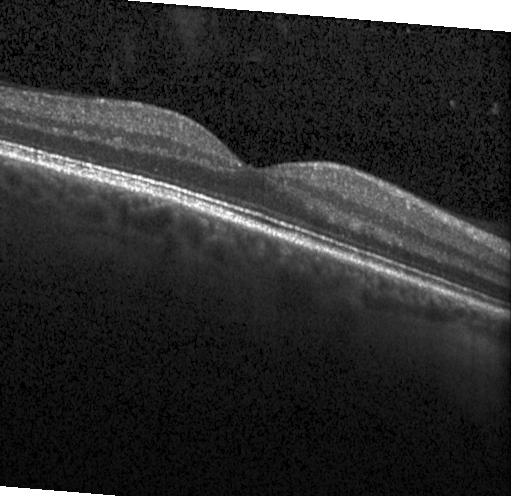
Retinal OCT cross-section. Diagnosis: no CNV, DME, or drusen.